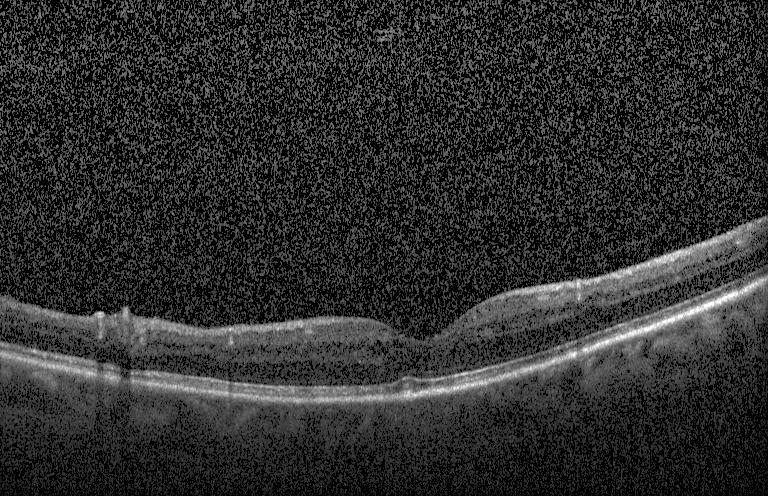
Acquired on a Heidelberg Spectralis; centered on the fovea; optical coherence tomography scan; SD-OCT.
No evidence of CNV, DME, or drusen.